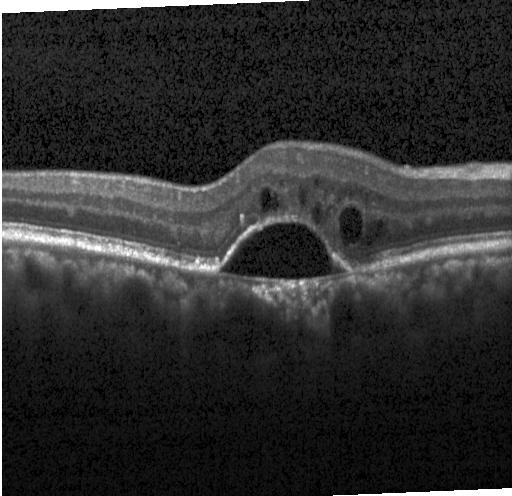
Retinal OCT cross-section, spectral-domain OCT, Heidelberg Spectralis OCT system
Finding: choroidal neovascularization.